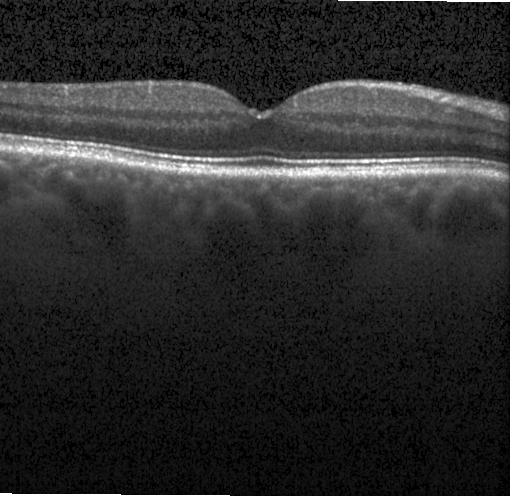
Spectral-domain OCT, acquired on a Heidelberg Spectralis, centered on the fovea, retinal OCT cross-section. Impression: no evidence of CNV, DME, or drusen.